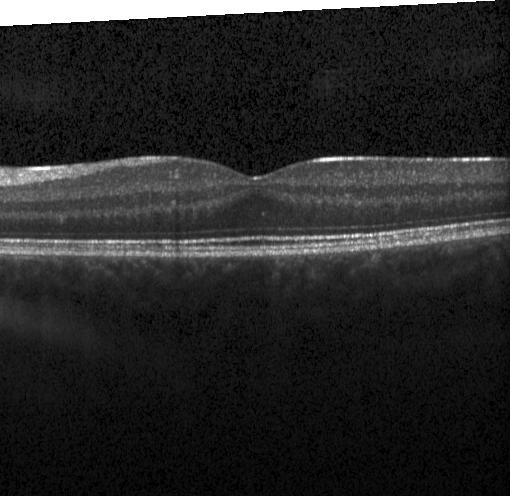

Retinal OCT cross-section. Assessment: no evidence of choroidal neovascularization, diabetic macular edema, or drusen.